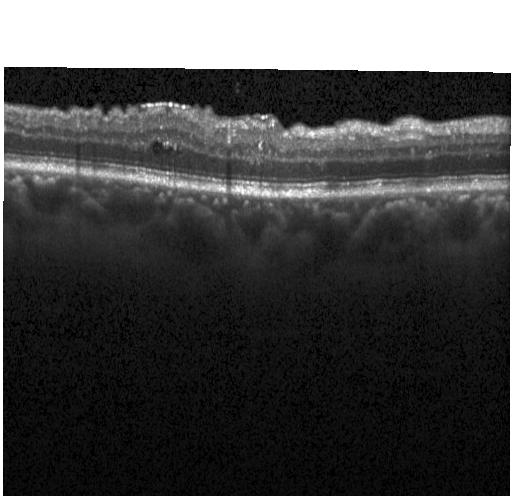
Impression: DME.